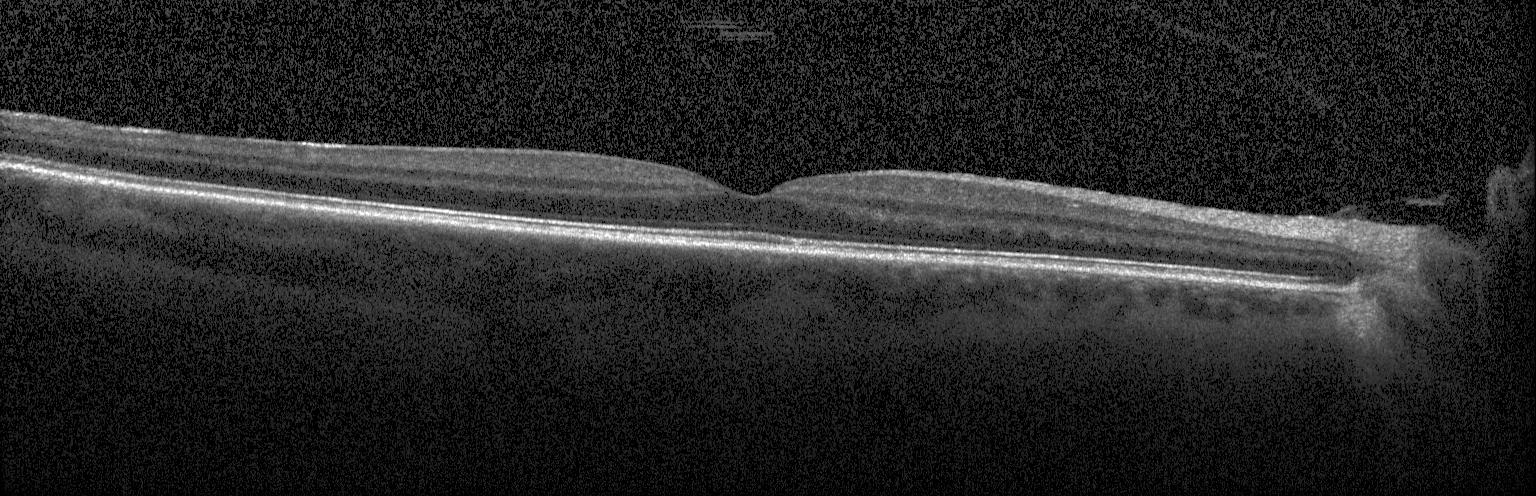

The scan shows no choroidal neovascularization, diabetic macular edema, or drusen.